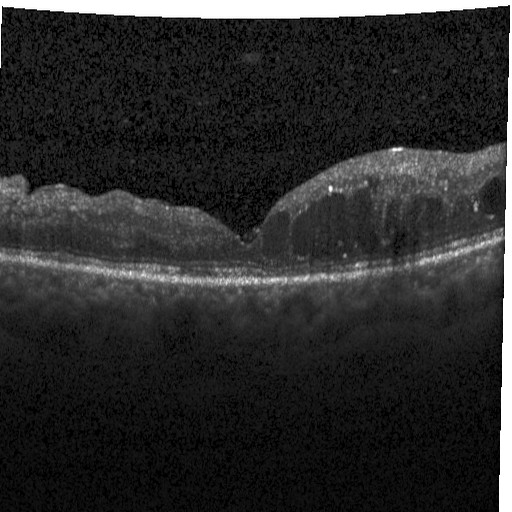
Impression: diabetic macular edema.